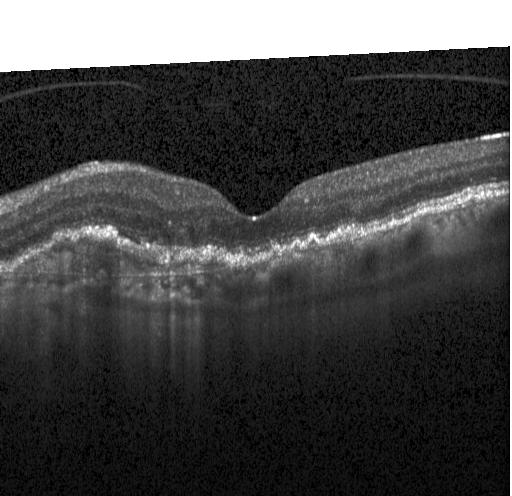

Impression: a choroidal neovascular membrane.